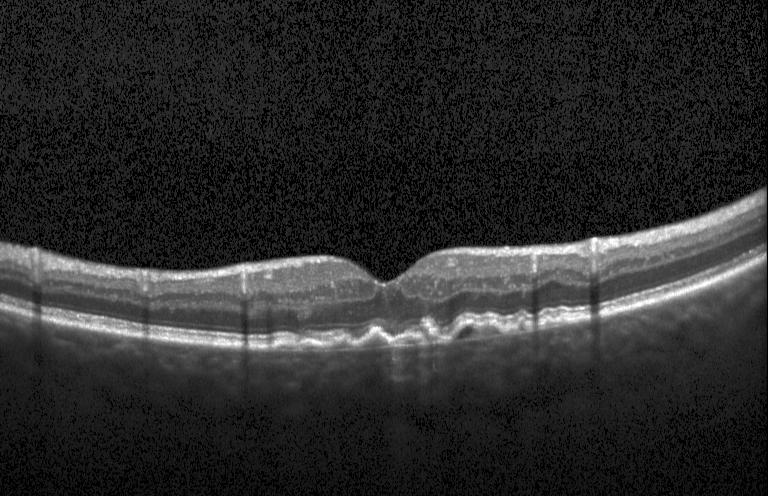
Retinal OCT cross-section · spectral-domain OCT · fovea-centered · Heidelberg Spectralis OCT system
Finding: drusen.